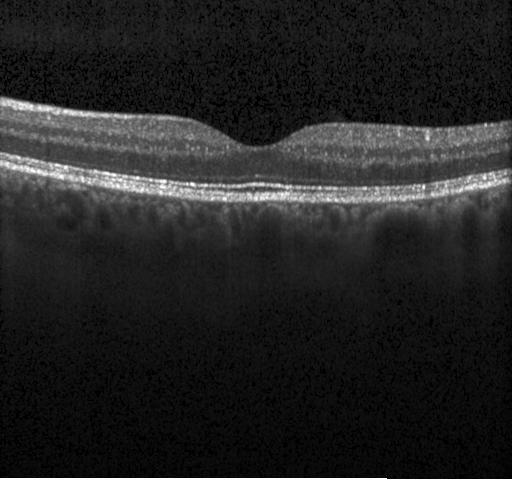 OCT finding: no choroidal neovascularization, diabetic macular edema, or drusen.